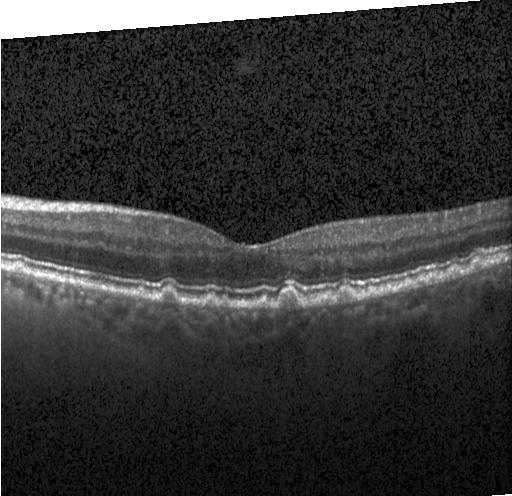 Diagnosis: sub-RPE drusenoid deposits.